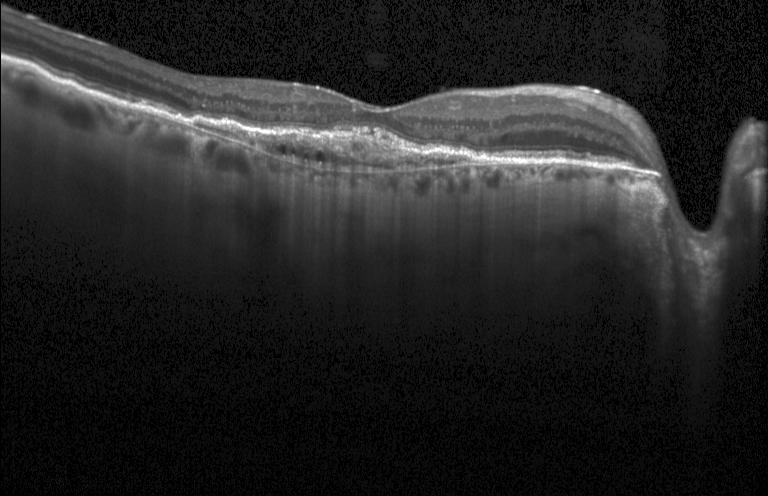 Retinal OCT B-scan.
Finding: CNV.